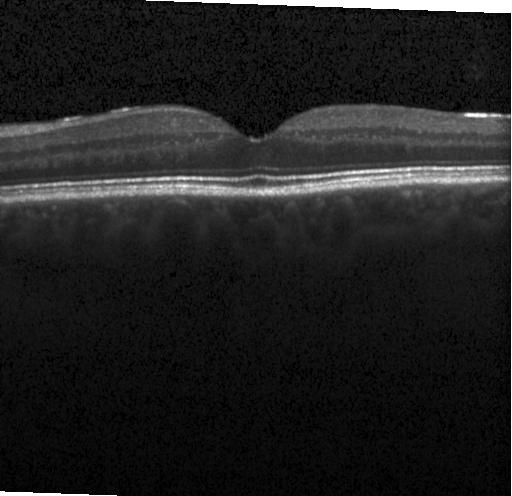
OCT B-scan · fovea-centered · Heidelberg Spectralis OCT system.
OCT finding: no CNV, no DME, and no drusen.